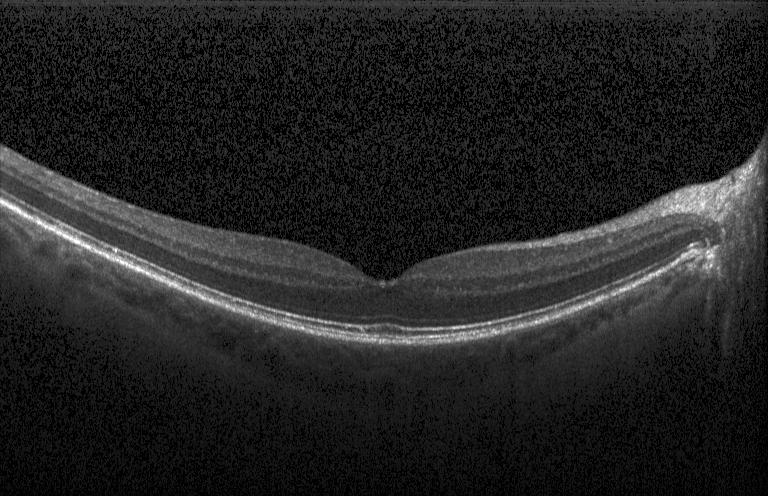
Optical coherence tomography B-scan.
This B-scan demonstrates neither choroidal neovascularization, diabetic macular edema, nor drusen.